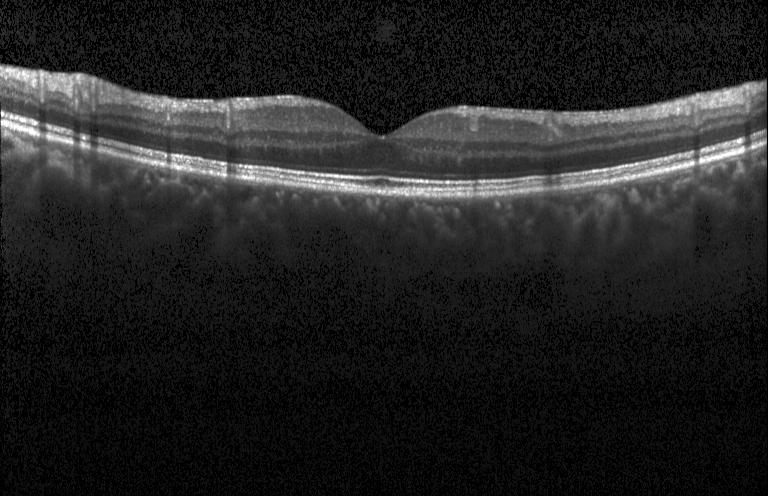

Horizontal scan through the fovea. SD-OCT. Heidelberg Spectralis OCT system. Optical coherence tomography scan — Diagnosis: no choroidal neovascularization, diabetic macular edema, or drusen.